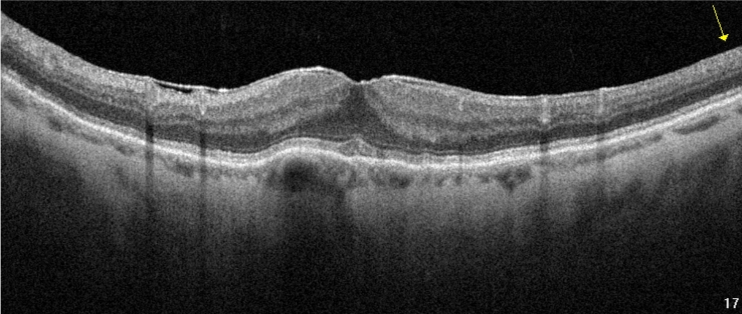
Retinal OCT B-scan — Impression: age-related macular degeneration.